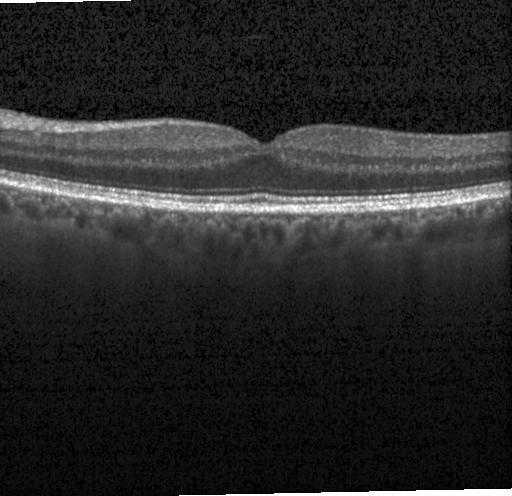 Retinal OCT B-scan — The scan shows neither choroidal neovascularization, diabetic macular edema, nor drusen.